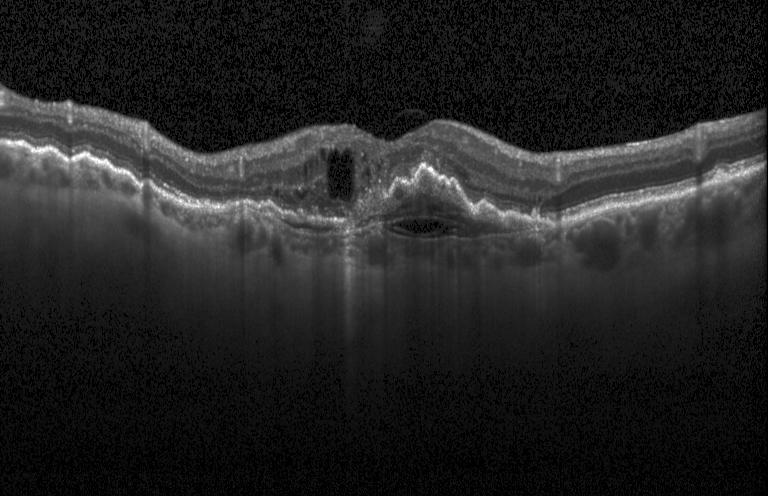
The scan shows a choroidal neovascular membrane.